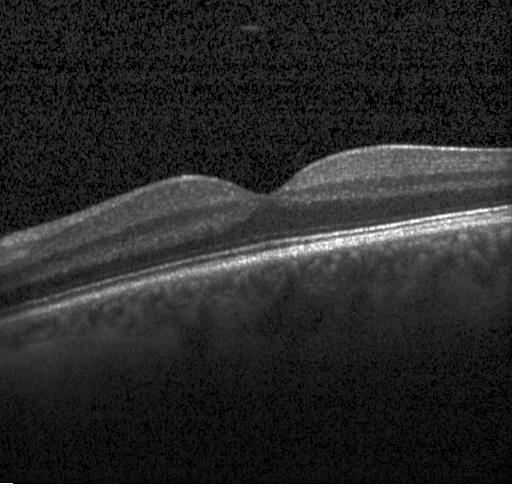

Through the macula · Heidelberg Spectralis OCT system · retinal OCT cross-section — Dx: no CNV, DME, or drusen.